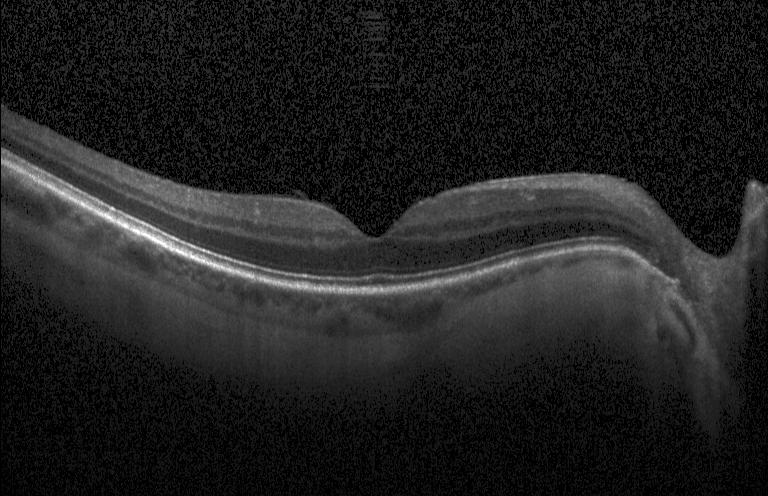
Assessment: no choroidal neovascularization, no diabetic macular edema, and no drusen.